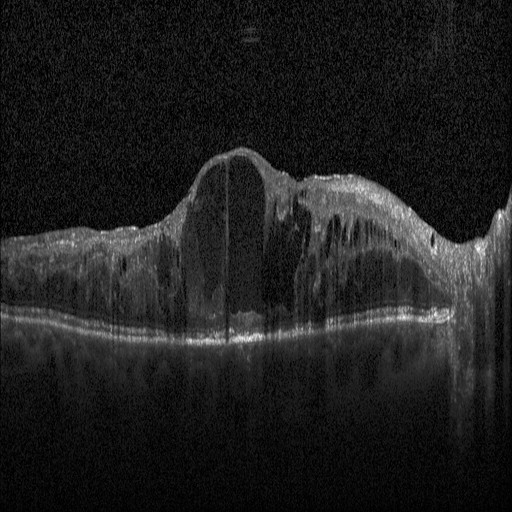

SD-OCT, retinal OCT cross-section, macular scan, instrument: Heidelberg Spectralis
Dx: diabetic macular edema.